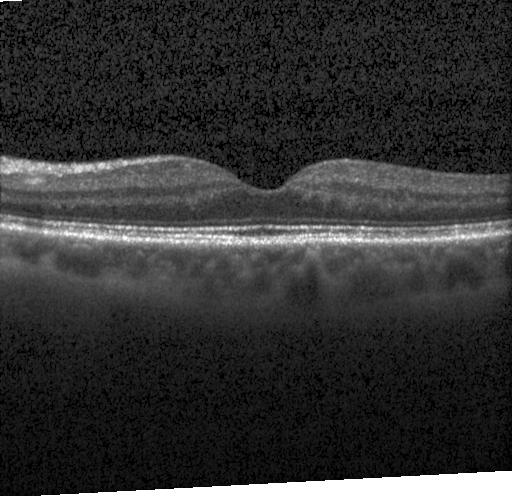

Optical coherence tomography B-scan.
No evidence of CNV, DME, or drusen.